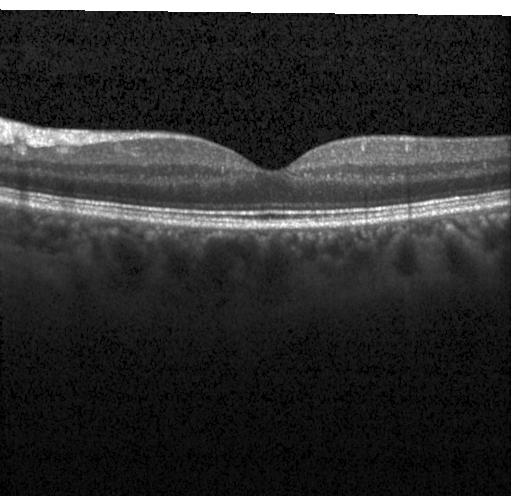 Acquired on a Heidelberg Spectralis; optical coherence tomography B-scan — Diagnosis: no choroidal neovascularization, no diabetic macular edema, and no drusen.